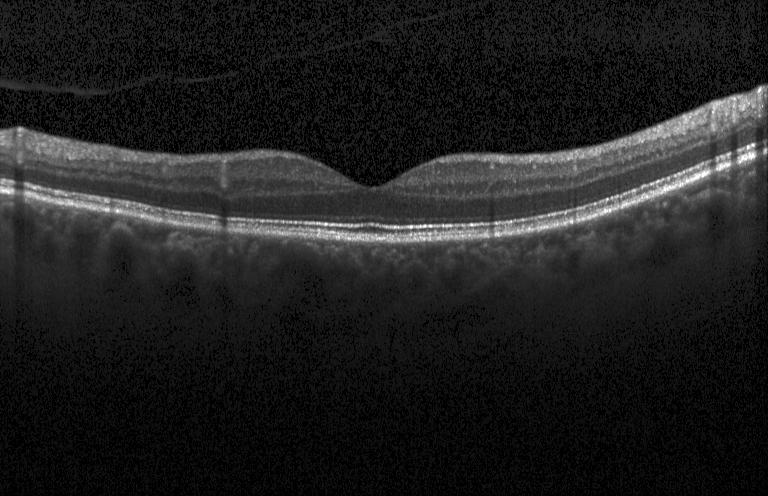
Finding: no evidence of choroidal neovascularization, diabetic macular edema, or drusen.